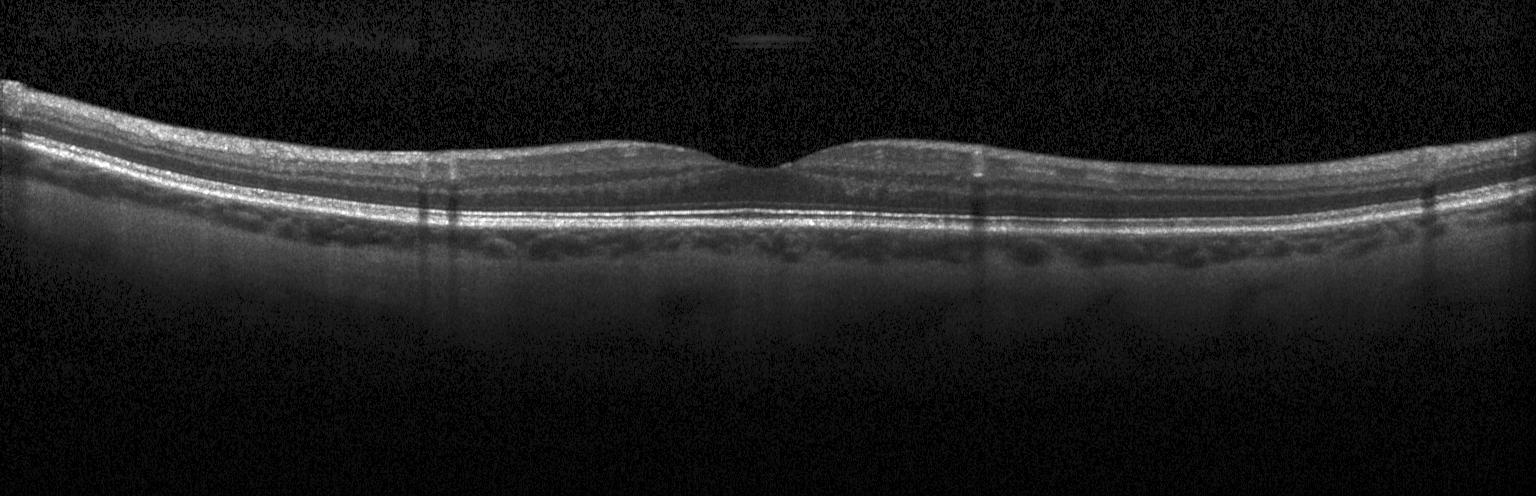 Retinal OCT B-scan, fovea-centered, acquired on a Heidelberg Spectralis — Finding: no choroidal neovascularization, no diabetic macular edema, and no drusen.